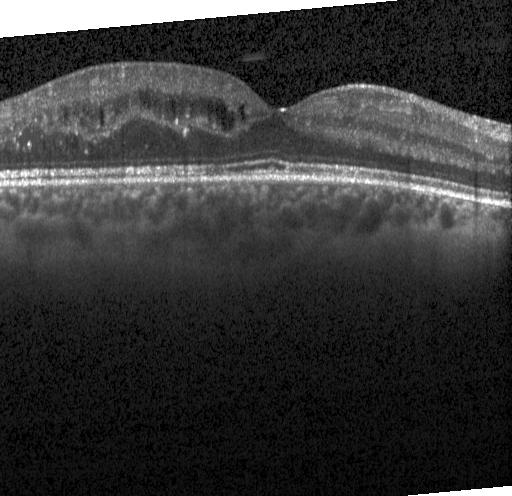

OCT finding: diabetic macular edema.